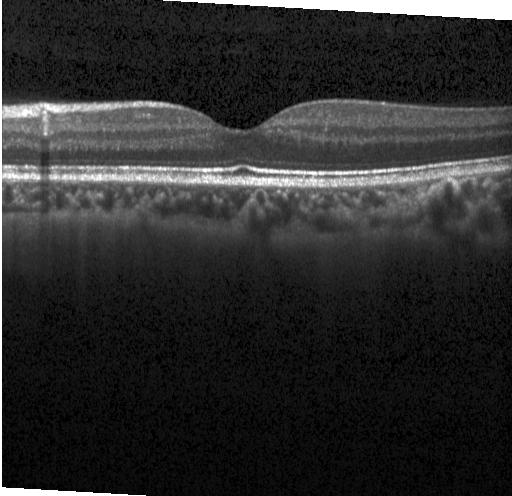 Macular scan · acquired on a Heidelberg Spectralis · optical coherence tomography scan · spectral-domain optical coherence tomography. No CNV, no DME, and no drusen.